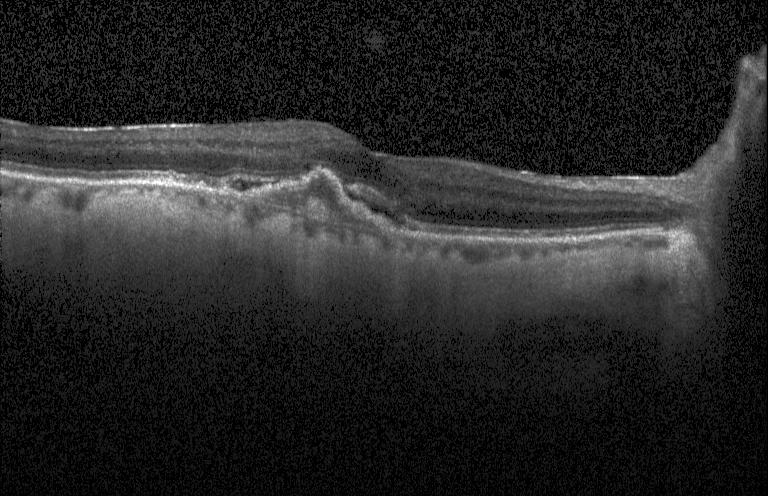

OCT B-scan — Impression: CNV.